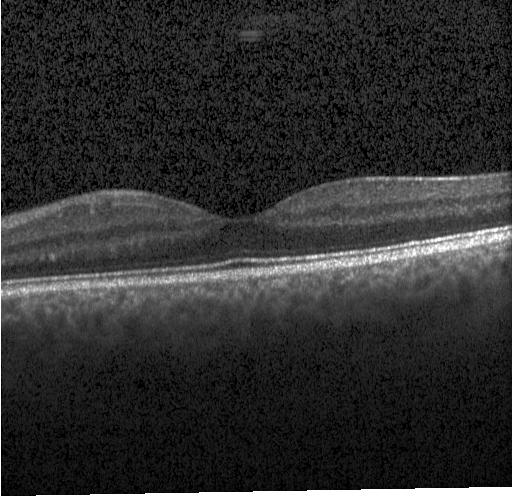 Retinal OCT cross-section showing no CNV, no DME, and no drusen.